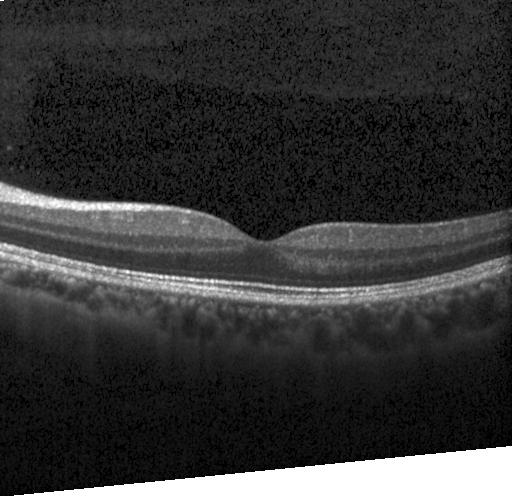

Heidelberg Spectralis; optical coherence tomography scan; macular scan.
Finding: no choroidal neovascularization, no diabetic macular edema, and no drusen.